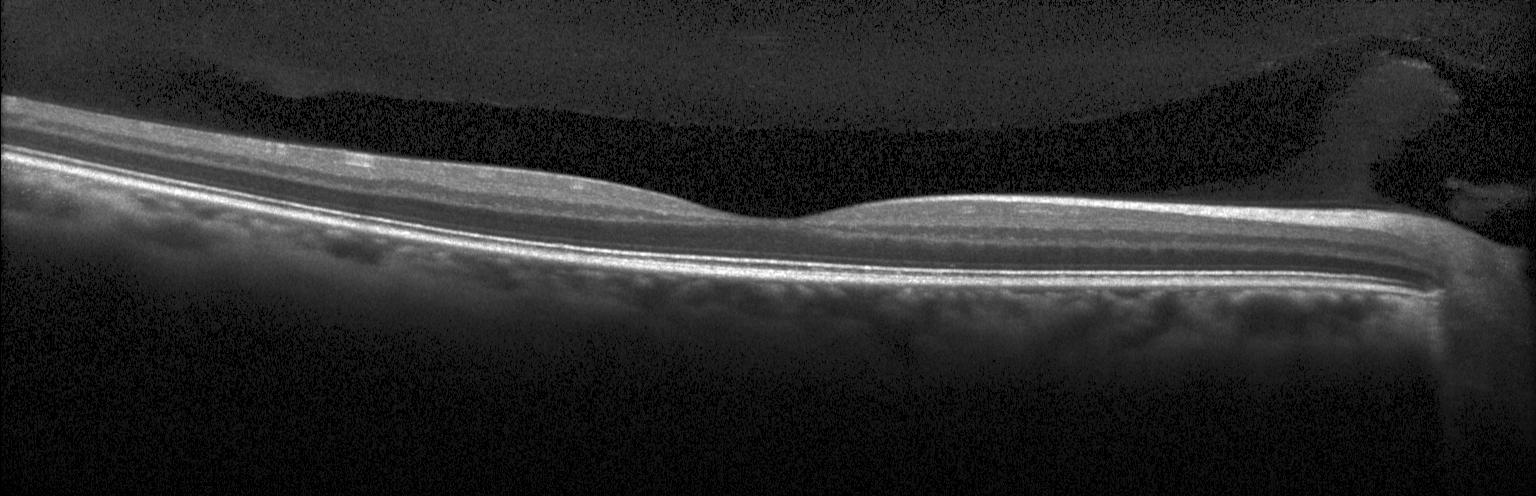
Spectral-domain optical coherence tomography. Retinal OCT B-scan
No evidence of choroidal neovascularization, diabetic macular edema, or drusen.